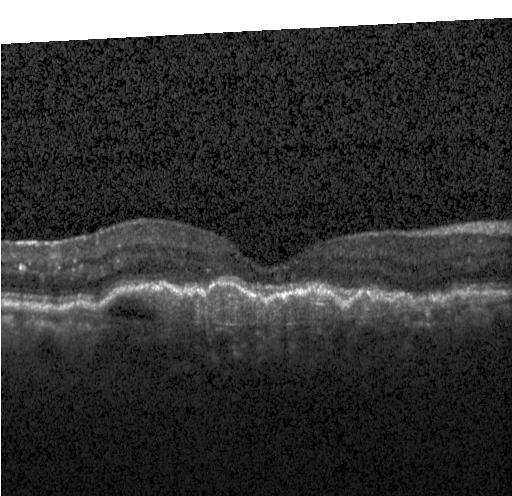

Diagnosis: CNV.